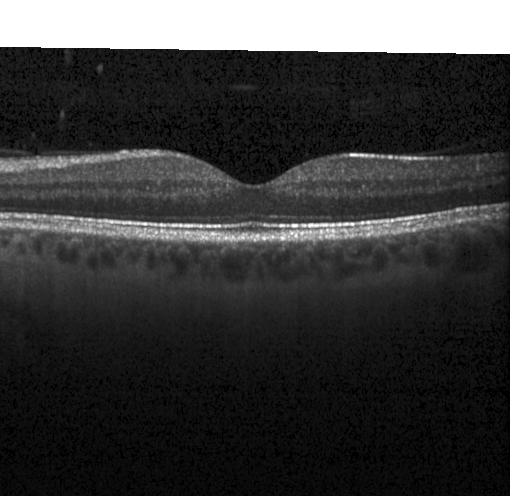
Optical coherence tomography scan
Dx: no evidence of choroidal neovascularization, diabetic macular edema, or drusen.